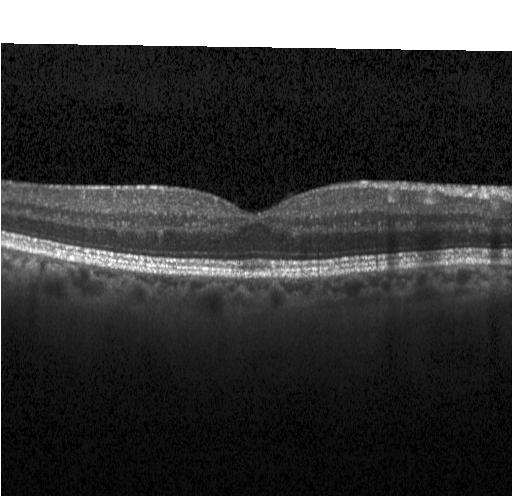

Through the macula. Optical coherence tomography scan
Impression: no CNV, DME, or drusen.